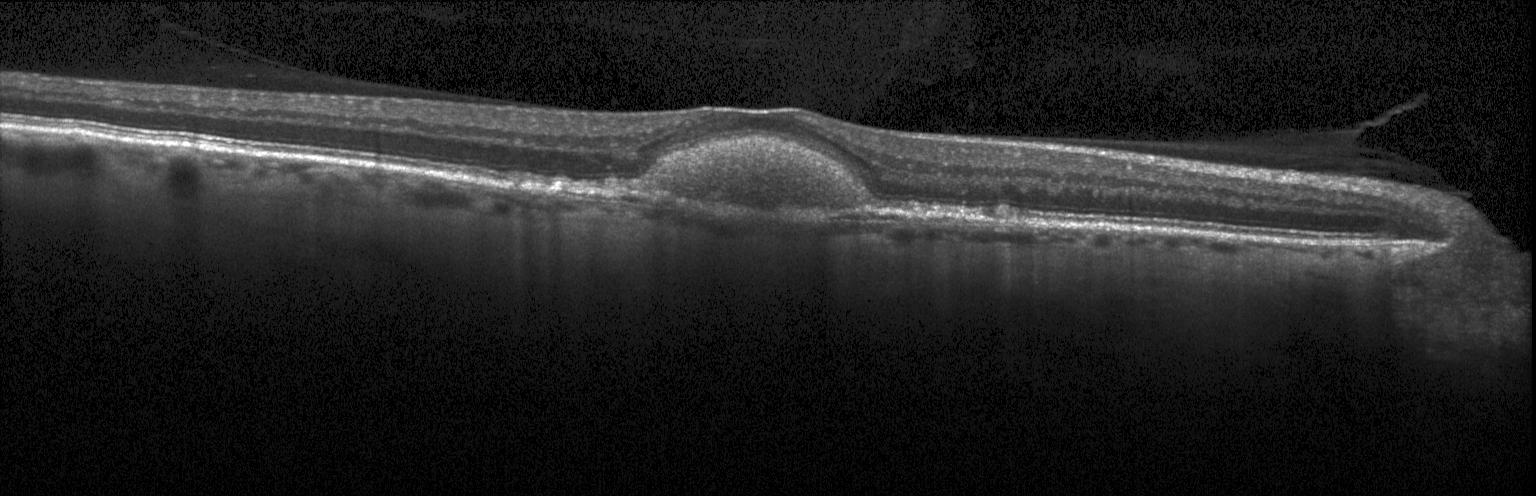

Finding: a choroidal neovascular membrane.